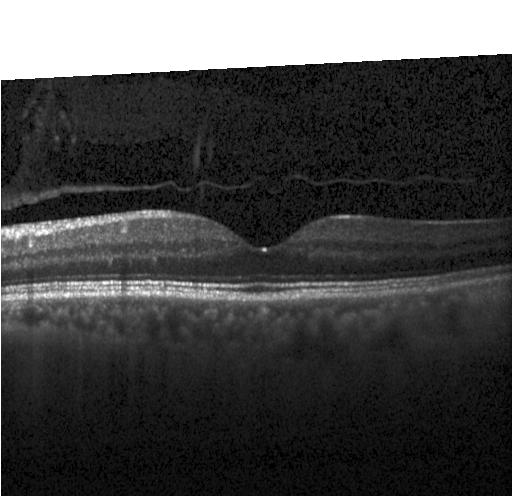 Impression: no evidence of choroidal neovascularization, diabetic macular edema, or drusen.